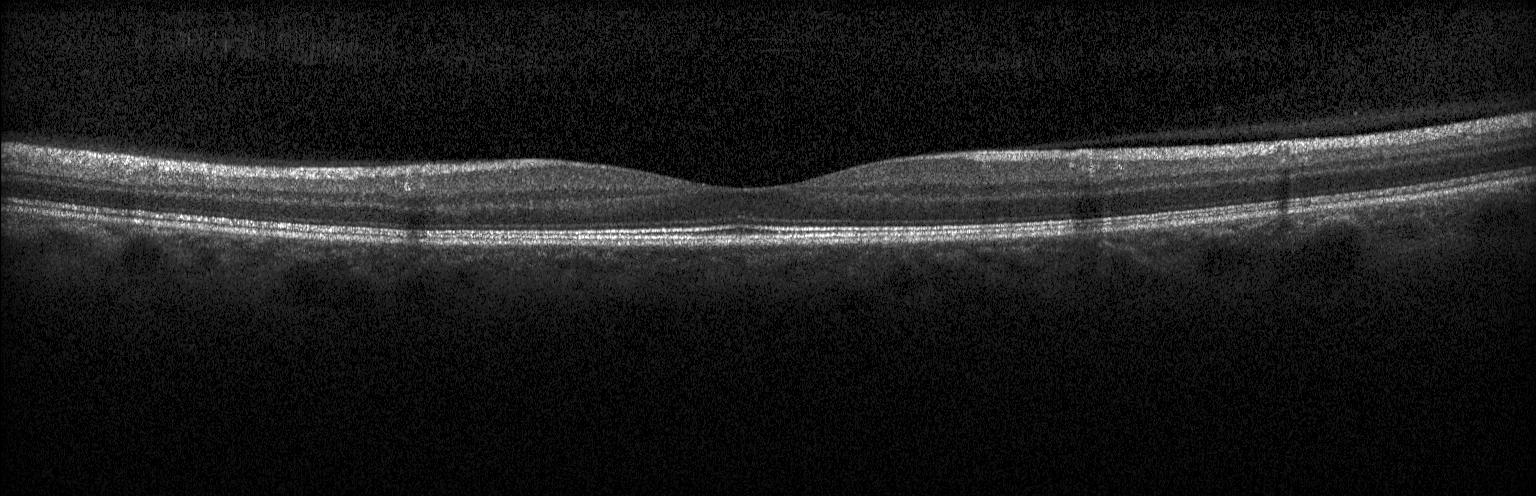

OCT finding: no choroidal neovascularization, no diabetic macular edema, and no drusen.